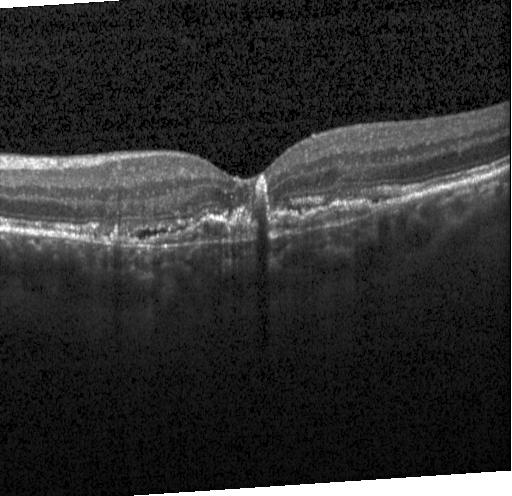 Heidelberg Spectralis OCT system, optical coherence tomography B-scan
Diagnosis: choroidal neovascularization (CNV).